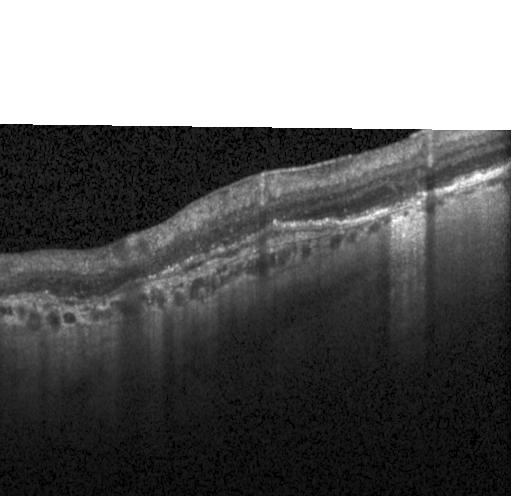 Fovea-centered, spectral-domain optical coherence tomography, acquired on a Heidelberg Spectralis, retinal OCT B-scan
Macular OCT: a choroidal neovascular membrane.